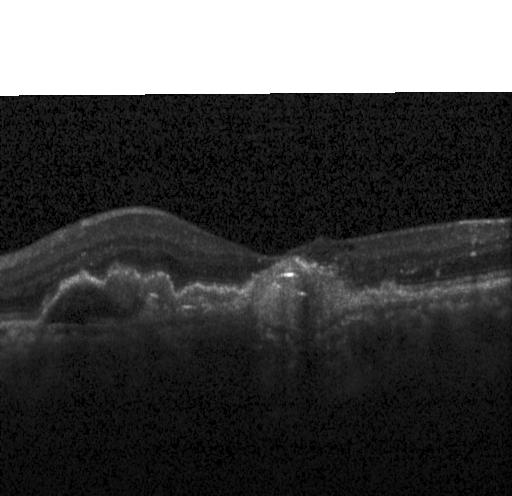 Macular scan; optical coherence tomography B-scan. Finding: a choroidal neovascular membrane.